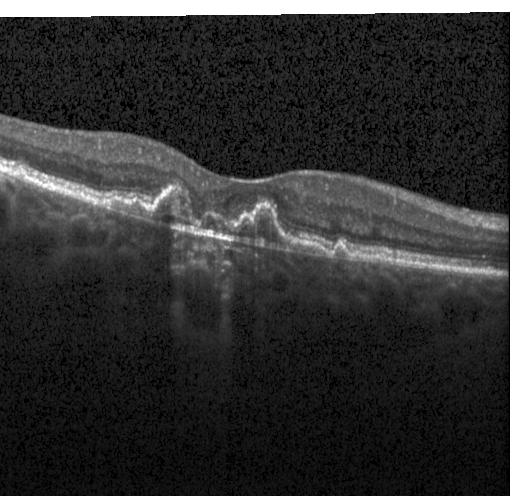 Centered on the fovea, optical coherence tomography scan.
Assessment: a choroidal neovascular membrane.